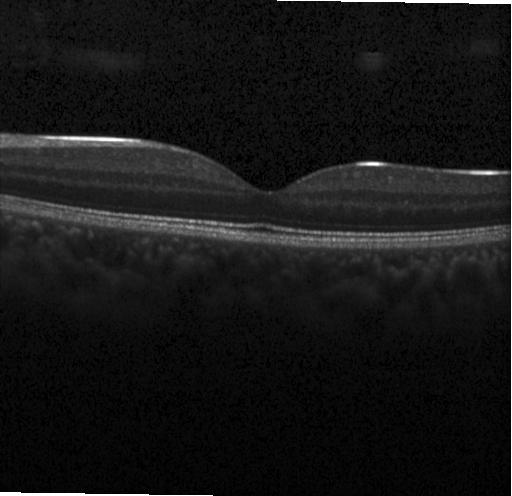
OCT finding: no evidence of CNV, DME, or drusen.